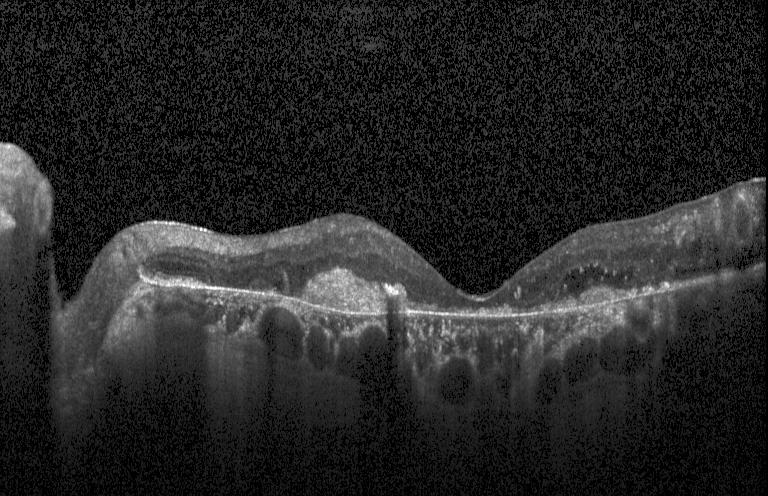
Optical coherence tomography scan — The scan shows choroidal neovascularization (CNV).